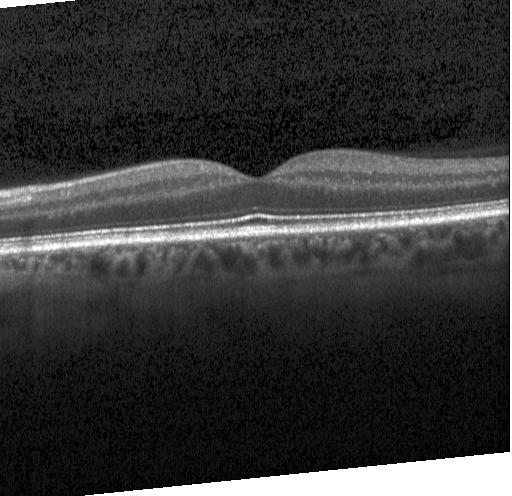 Impression: no choroidal neovascularization, diabetic macular edema, or drusen.